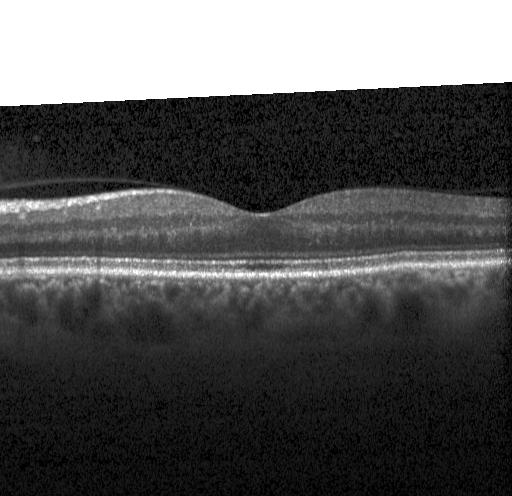
OCT scan showing no choroidal neovascularization, no diabetic macular edema, and no drusen.